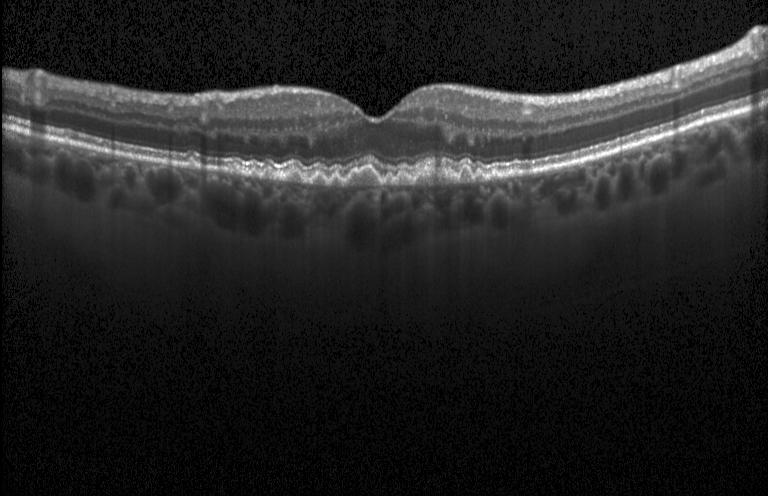

OCT line scan, SD-OCT.
The scan shows sub-RPE drusenoid deposits.